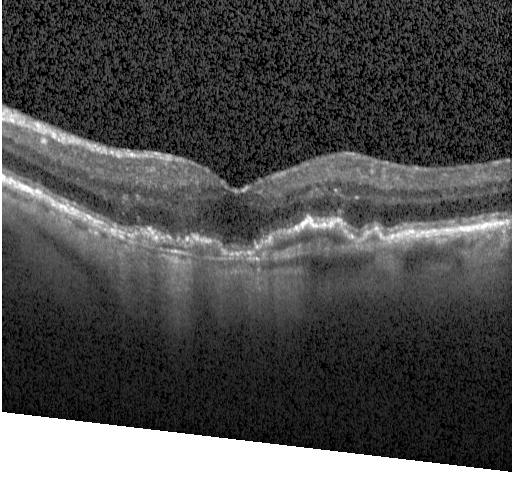 Dx: choroidal neovascularization.